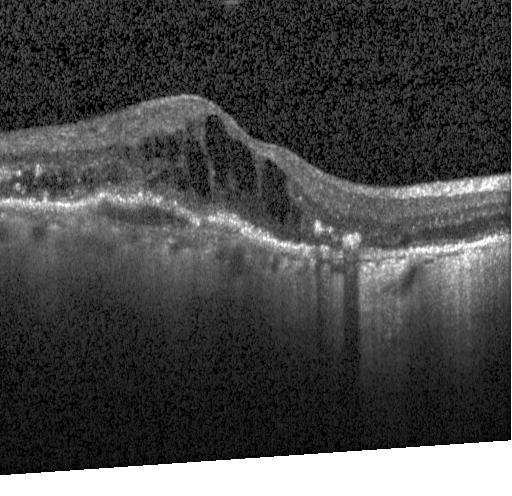

SD-OCT · macular scan · Heidelberg Spectralis OCT system · optical coherence tomography B-scan. Impression: CNV.